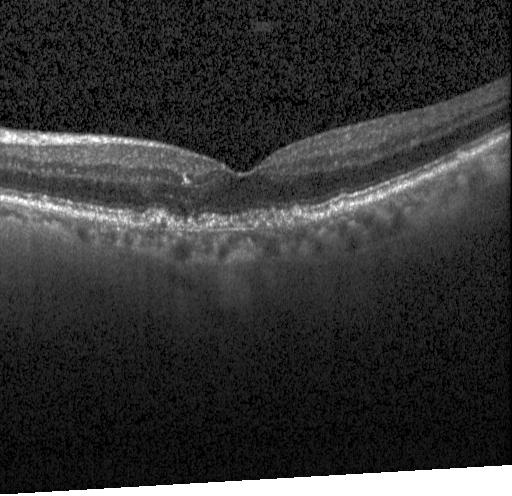
Retinal OCT cross-section — Impression: drusen.